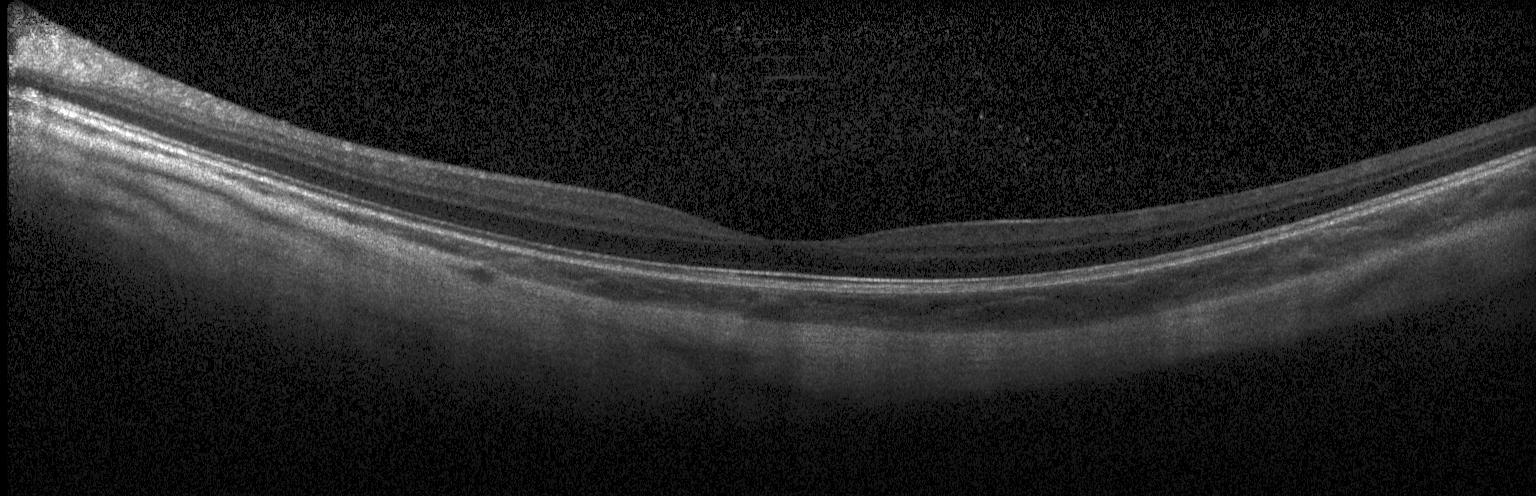

Acquired on a Heidelberg Spectralis · optical coherence tomography B-scan · spectral-domain OCT.
Finding: no evidence of choroidal neovascularization, diabetic macular edema, or drusen.